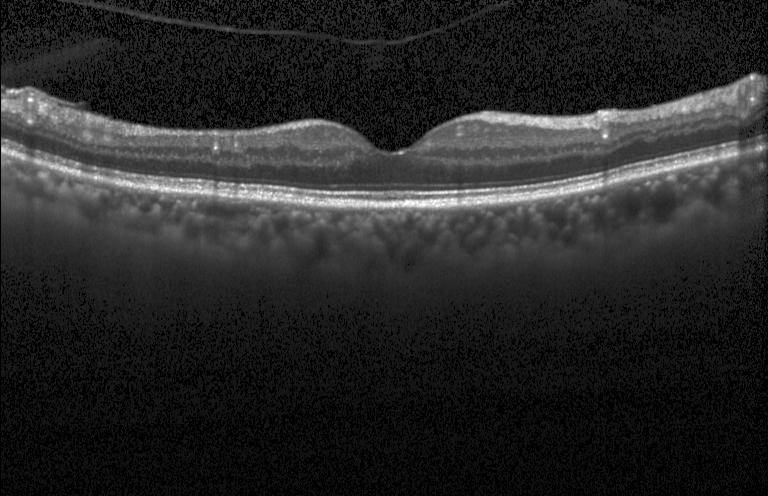 OCT line scan. Finding: no choroidal neovascularization, diabetic macular edema, or drusen.